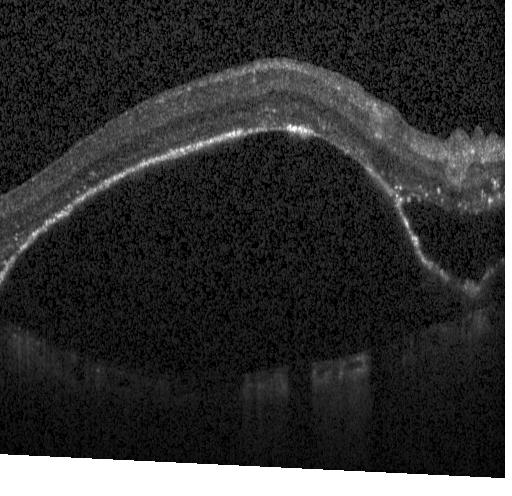

Dx: a choroidal neovascular membrane.